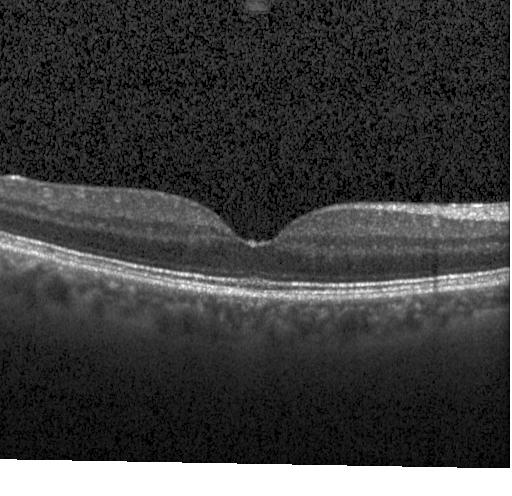 Retinal OCT cross-section; spectral-domain OCT. Impression: no evidence of choroidal neovascularization, diabetic macular edema, or drusen.